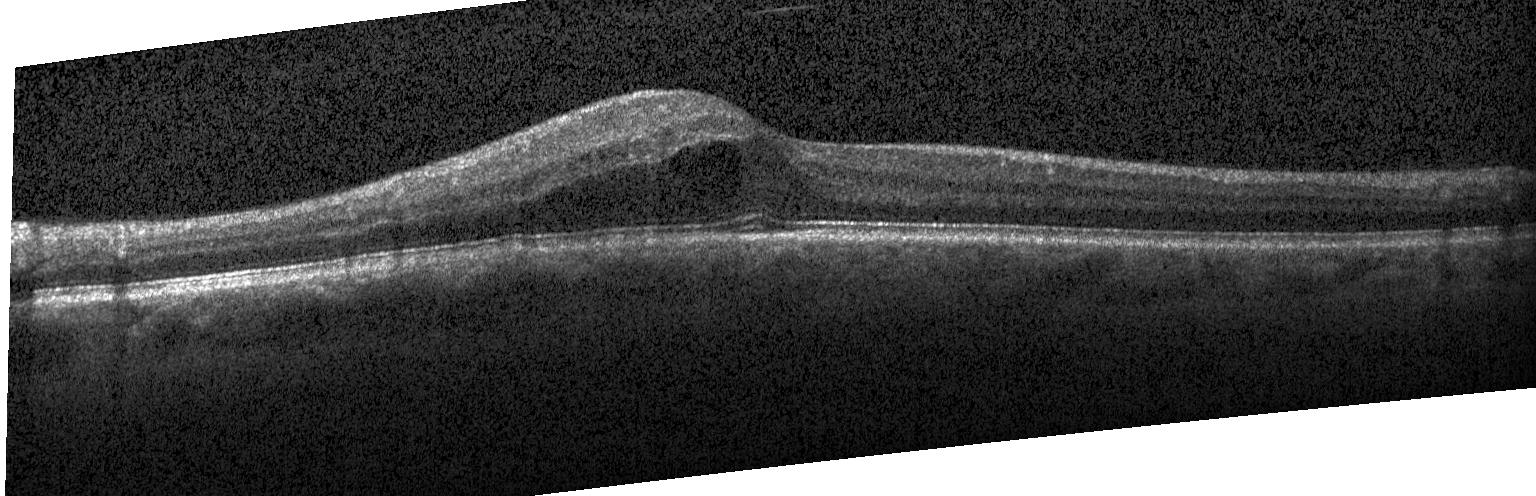 Heidelberg Spectralis; spectral-domain optical coherence tomography; optical coherence tomography B-scan
OCT finding: diabetic macular edema (DME).